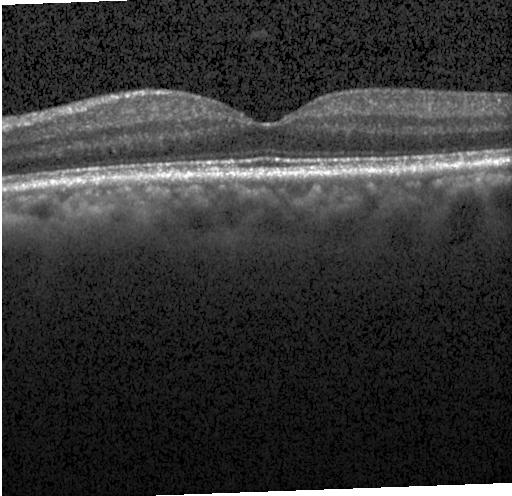 Impression: no choroidal neovascularization, diabetic macular edema, or drusen.